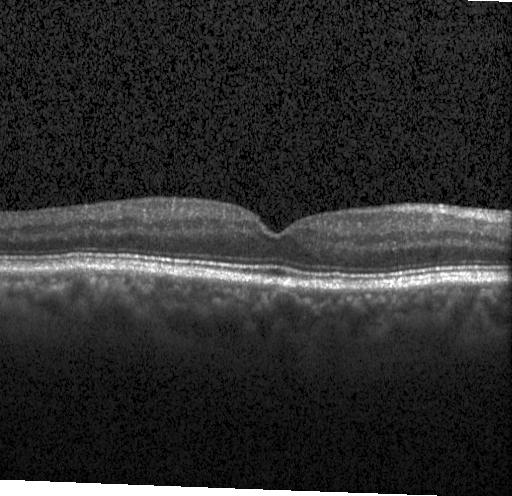
OCT line scan. Heidelberg Spectralis. SD-OCT — Diagnosis: neither CNV, DME, nor drusen.